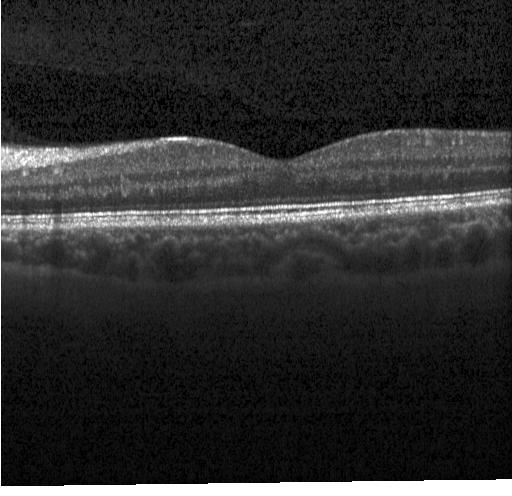 Diagnosis: no CNV, DME, or drusen.